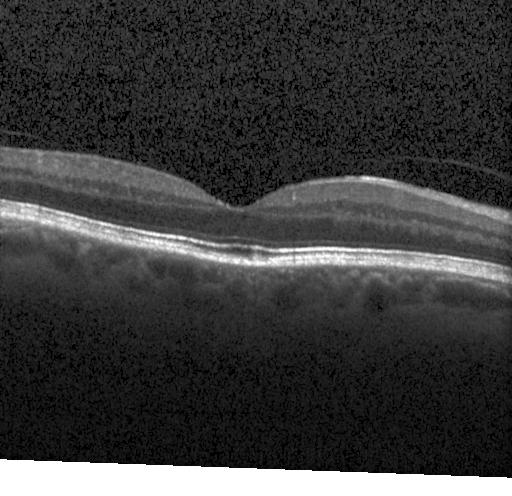

Retinal OCT B-scan. No evidence of choroidal neovascularization, diabetic macular edema, or drusen.